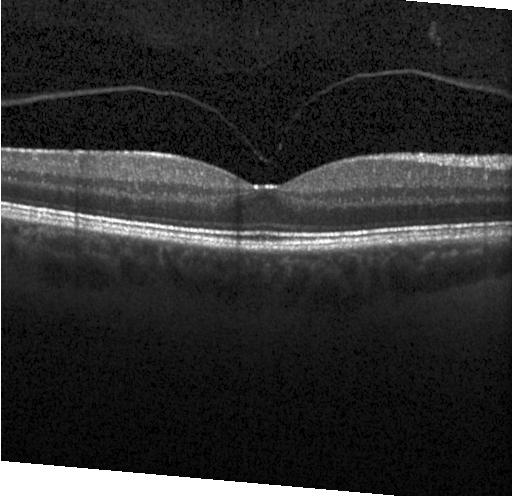

Macular OCT demonstrating no evidence of choroidal neovascularization, diabetic macular edema, or drusen.